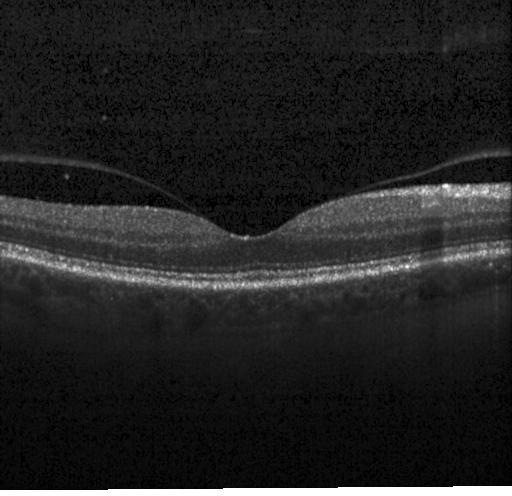

Retinal OCT B-scan. Centered on the fovea.
The scan shows no choroidal neovascularization, diabetic macular edema, or drusen.